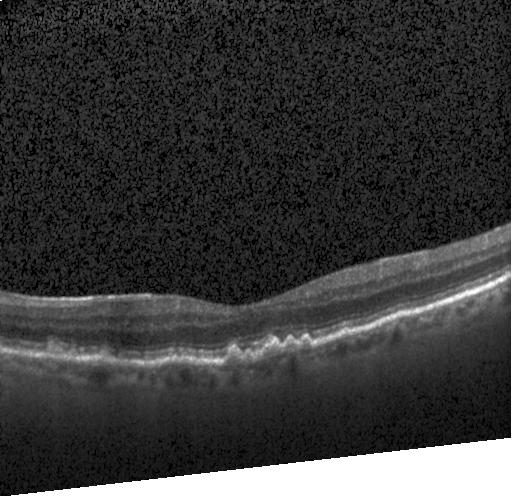
OCT B-scan, horizontal scan through the fovea, instrument: Heidelberg Spectralis — Finding: multiple drusen.